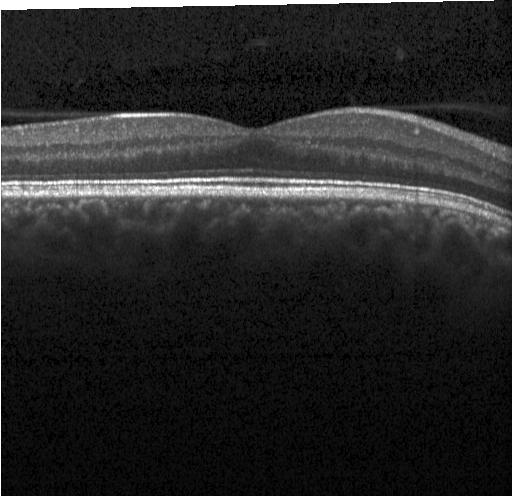
Acquired on a Heidelberg Spectralis, OCT B-scan, SD-OCT, fovea-centered — Diagnosis: no CNV, no DME, and no drusen.